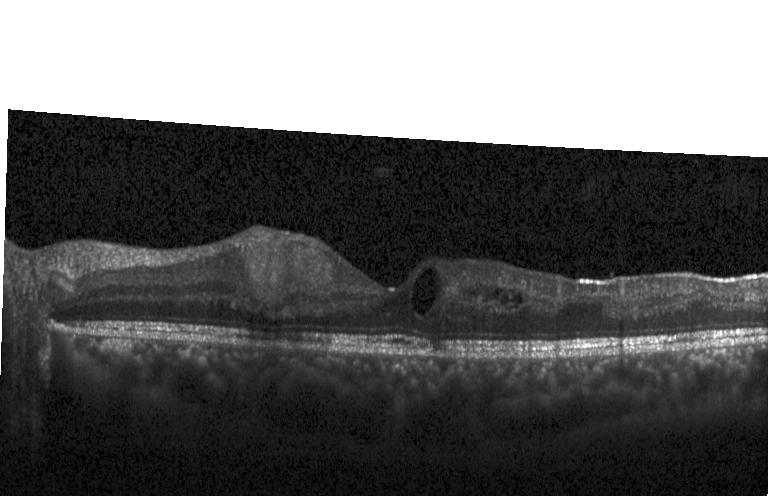
OCT line scan — Impression: diabetic macular edema (DME).